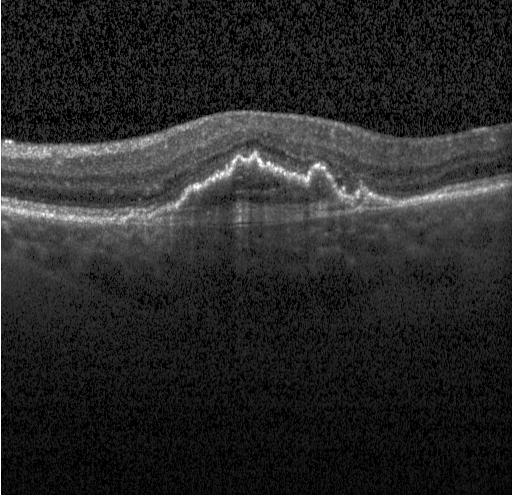
Impression: CNV.